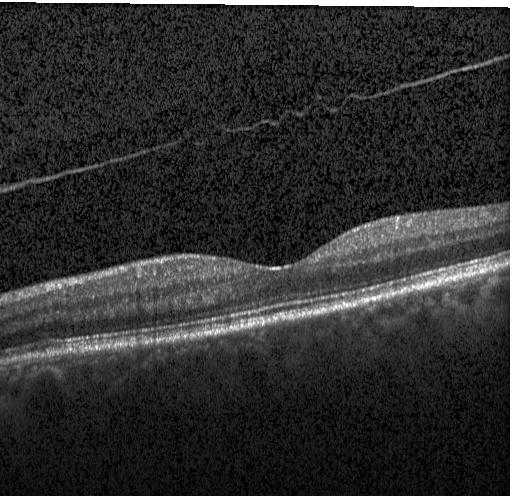

Macular OCT: neither choroidal neovascularization, diabetic macular edema, nor drusen.